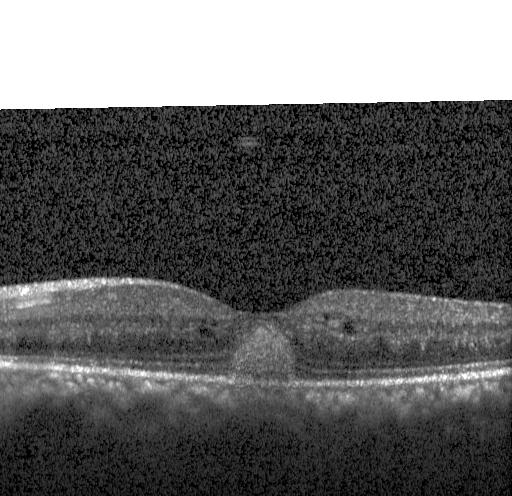
Horizontal scan through the fovea; spectral-domain OCT; retinal OCT B-scan
This B-scan demonstrates a choroidal neovascular membrane.